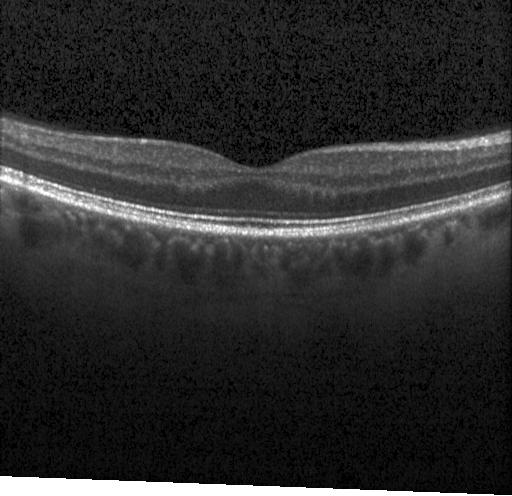
Acquired on a Heidelberg Spectralis; spectral-domain OCT; optical coherence tomography B-scan; centered on the fovea — Assessment: no CNV, no DME, and no drusen.